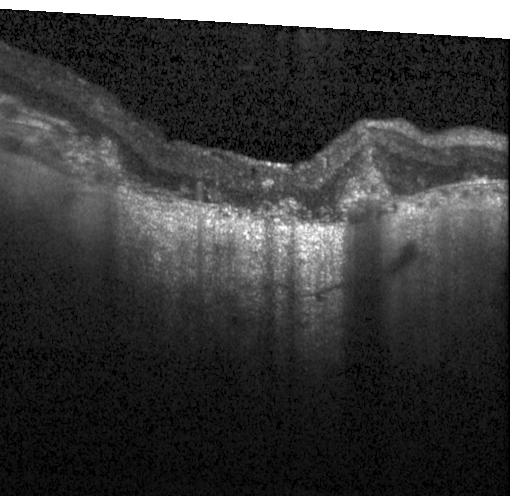
Centered on the fovea. Spectral-domain OCT. Optical coherence tomography scan. Instrument: Heidelberg Spectralis.
Macular OCT: CNV.